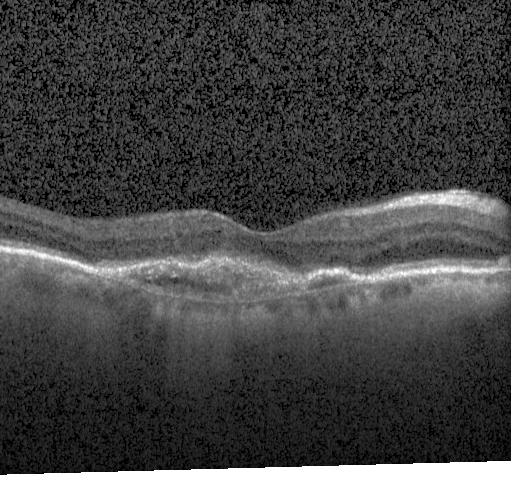 Dx: choroidal neovascularization.